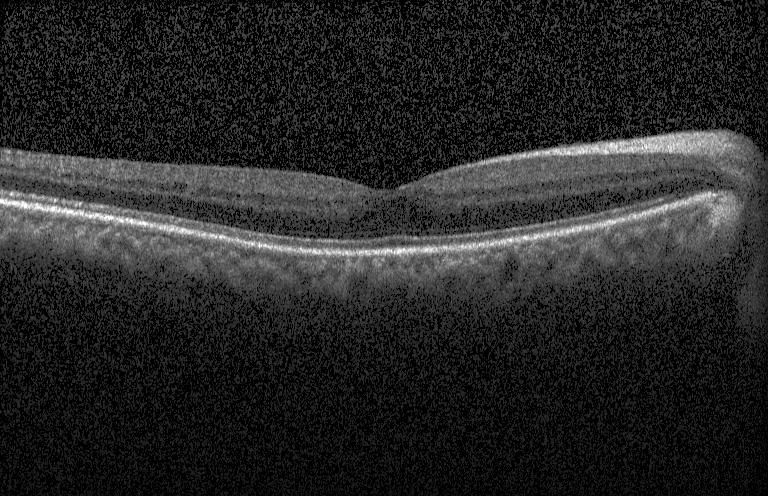
Horizontal scan through the fovea; spectral-domain optical coherence tomography; Heidelberg Spectralis OCT system; OCT line scan. This B-scan demonstrates no evidence of CNV, DME, or drusen.